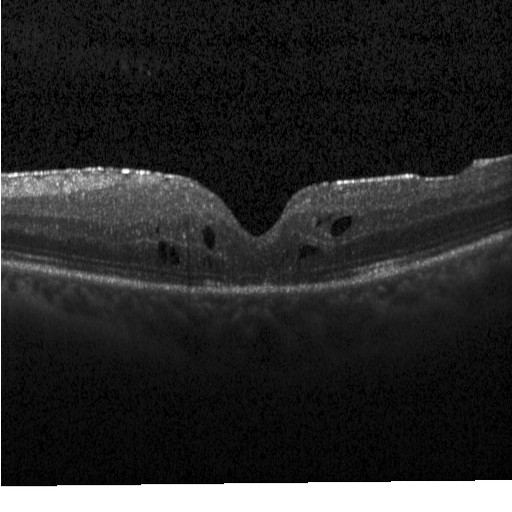

Diagnosis: DME.